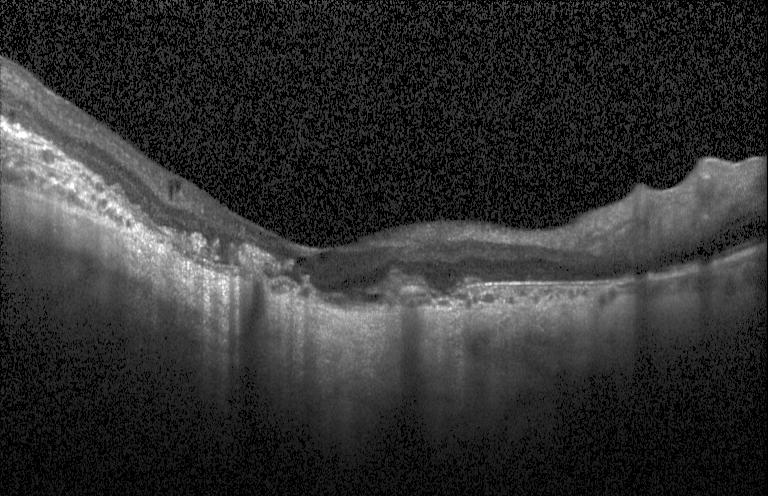
Retinal OCT cross-section. Spectral-domain OCT. Macular scan.
The scan shows choroidal neovascularization (CNV).